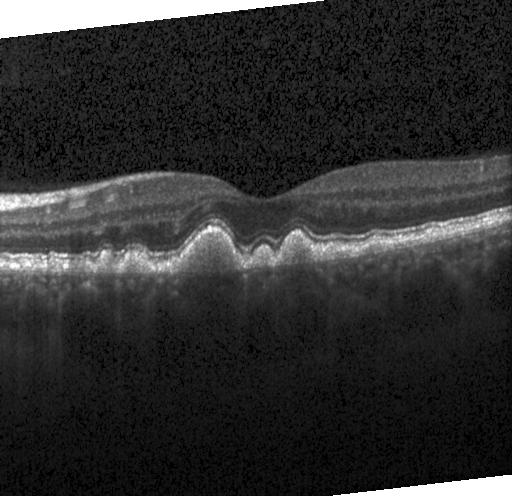

Instrument: Heidelberg Spectralis; retinal OCT cross-section; fovea-centered — Impression: multiple drusen.